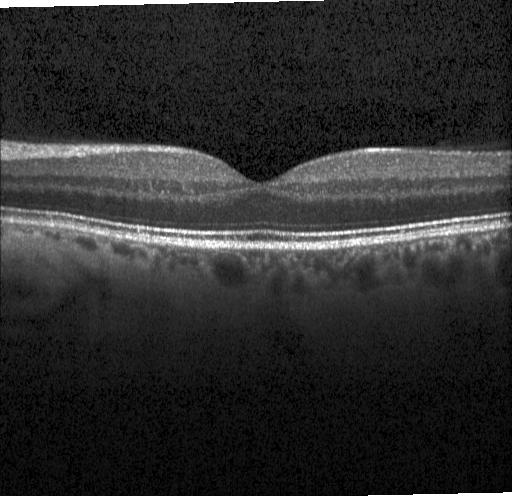
OCT B-scan
Neither choroidal neovascularization, diabetic macular edema, nor drusen.